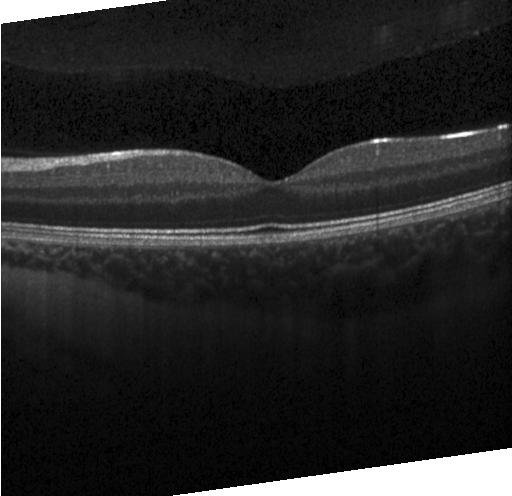
Retinal OCT B-scan — This B-scan demonstrates neither choroidal neovascularization, diabetic macular edema, nor drusen.